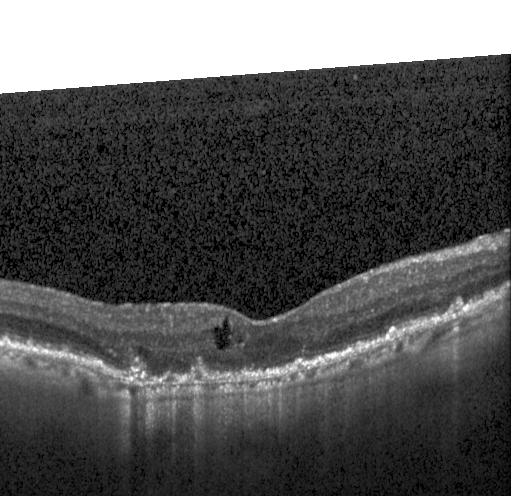

Retinal OCT cross-section showing a choroidal neovascular membrane.